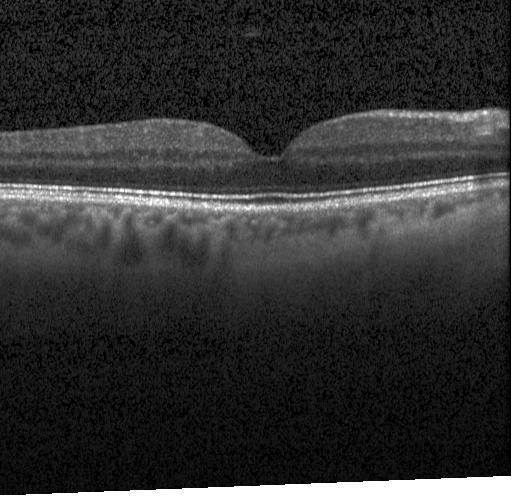 Impression: no CNV, no DME, and no drusen.